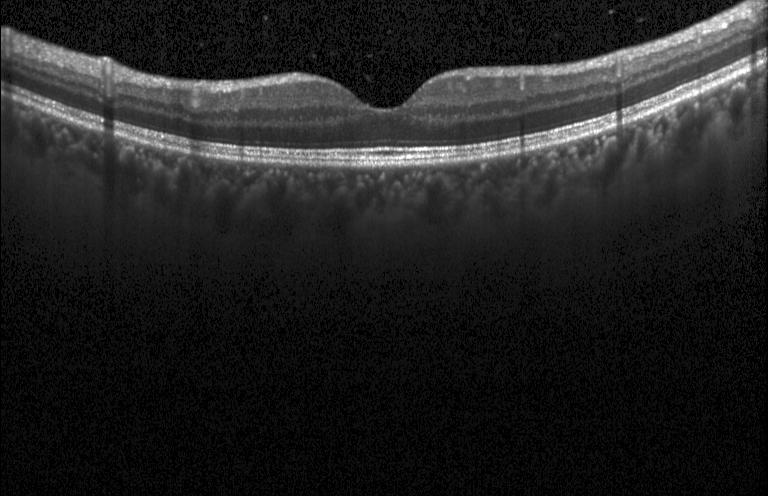

Spectral-domain OCT · optical coherence tomography scan · centered on the fovea · Heidelberg Spectralis OCT system.
OCT finding: no choroidal neovascularization, no diabetic macular edema, and no drusen.